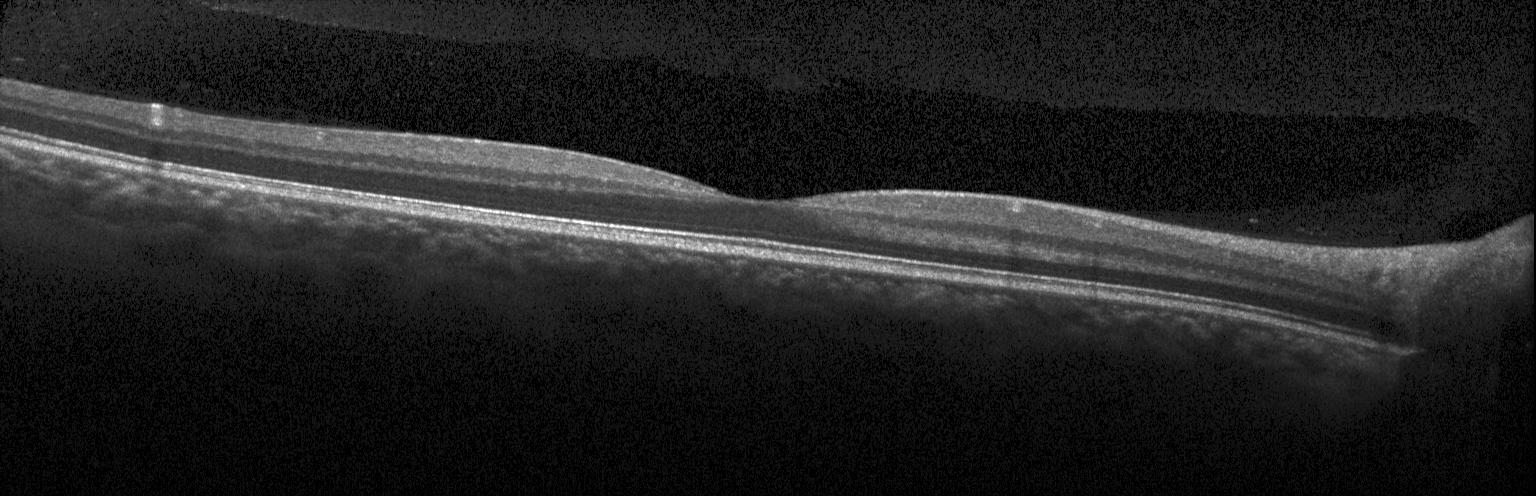 Retinal OCT cross-section showing neither choroidal neovascularization, diabetic macular edema, nor drusen.